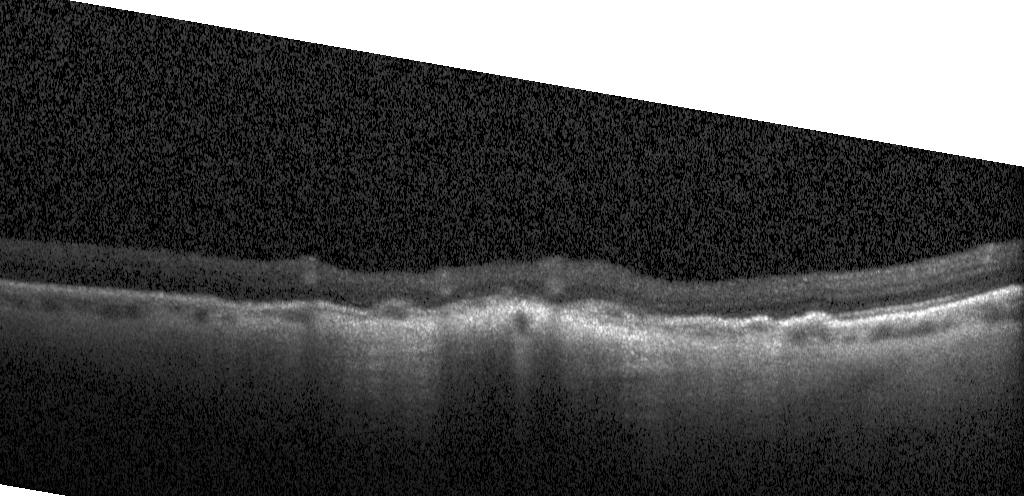
Acquired on a Heidelberg Spectralis. Retinal OCT cross-section. Fovea-centered. Spectral-domain optical coherence tomography. Finding: a choroidal neovascular membrane.